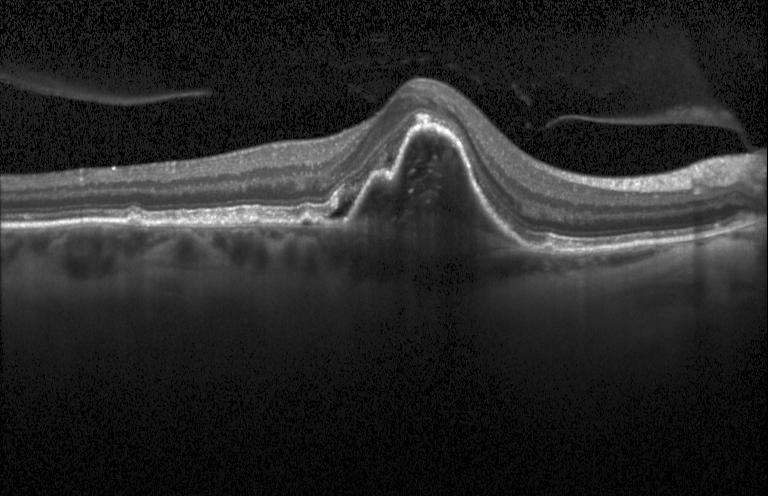 OCT B-scan. Instrument: Heidelberg Spectralis.
A choroidal neovascular membrane.